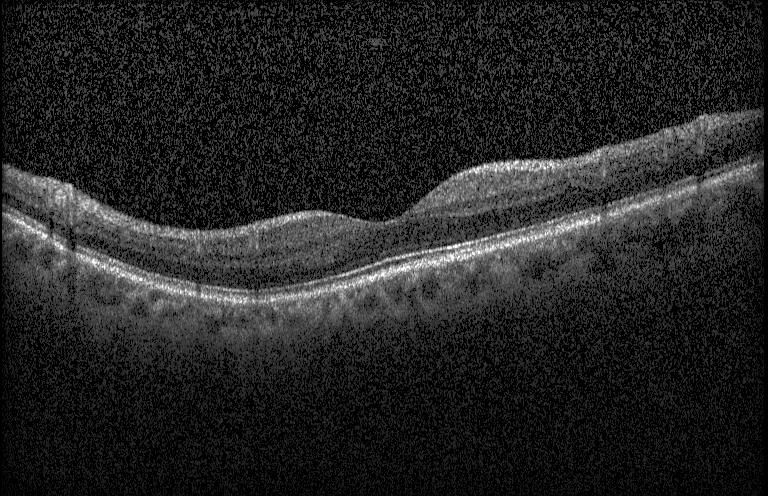 OCT line scan. Fovea-centered. Spectral-domain optical coherence tomography. Instrument: Heidelberg Spectralis.
OCT finding: no choroidal neovascularization, no diabetic macular edema, and no drusen.